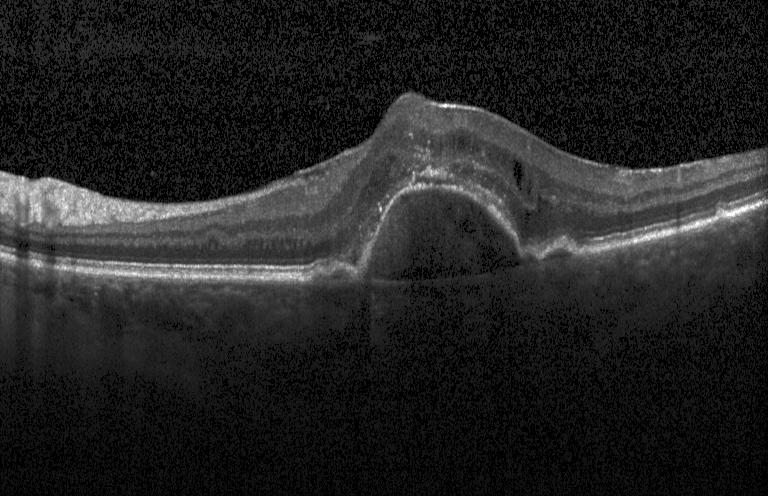

Spectral-domain OCT · acquired on a Heidelberg Spectralis · horizontal scan through the fovea · optical coherence tomography B-scan.
Impression: CNV.